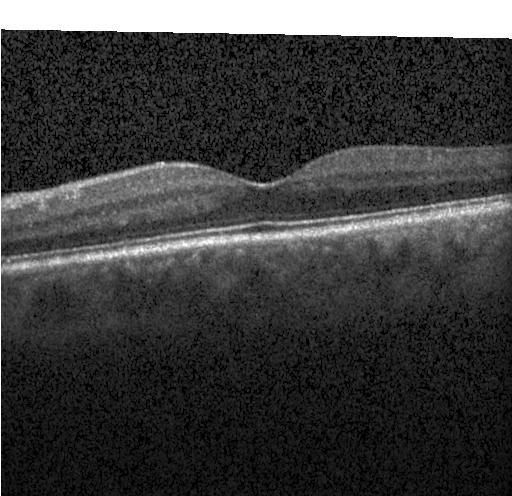
Instrument: Heidelberg Spectralis. Horizontal scan through the fovea. Optical coherence tomography scan. SD-OCT — Diagnosis: no choroidal neovascularization, no diabetic macular edema, and no drusen.